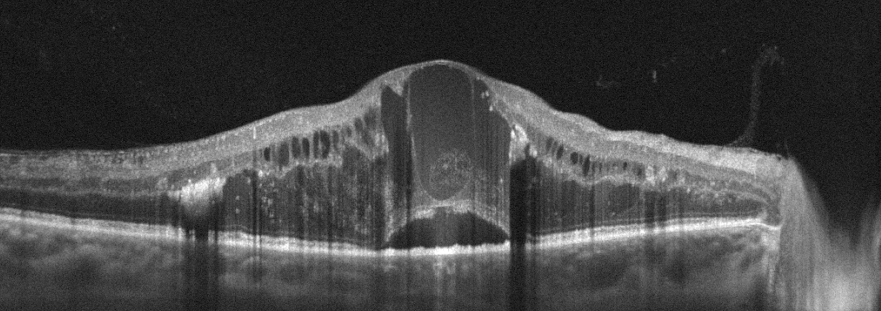
Optical coherence tomography scan. Diagnosis: diabetic macular edema.